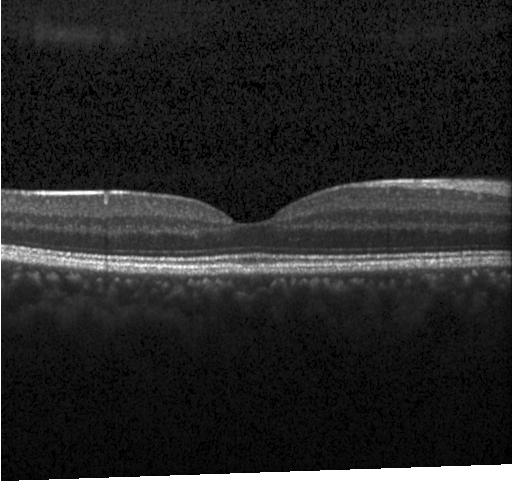
OCT finding: neither choroidal neovascularization, diabetic macular edema, nor drusen.